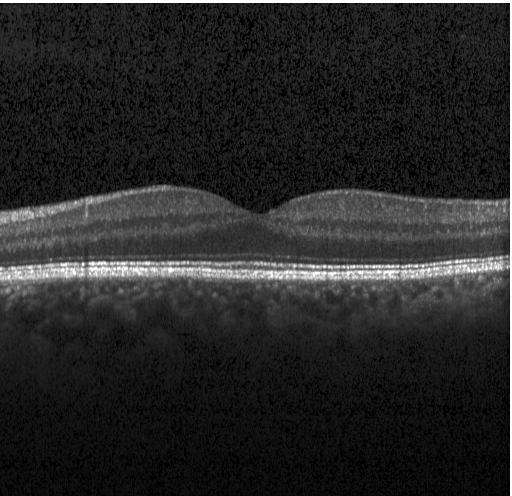
Retinal OCT B-scan. Horizontal scan through the fovea. Spectral-domain OCT — No choroidal neovascularization, diabetic macular edema, or drusen.